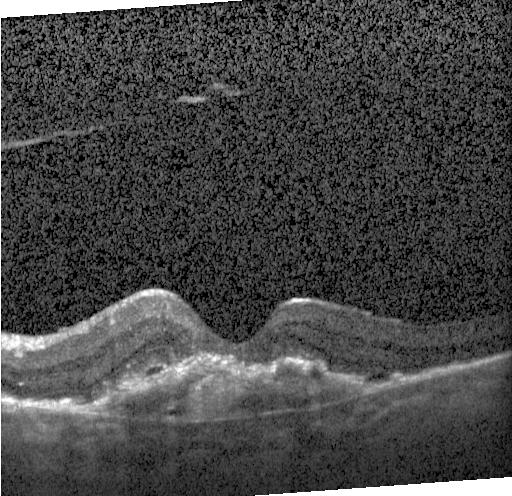
Diagnosis: CNV.